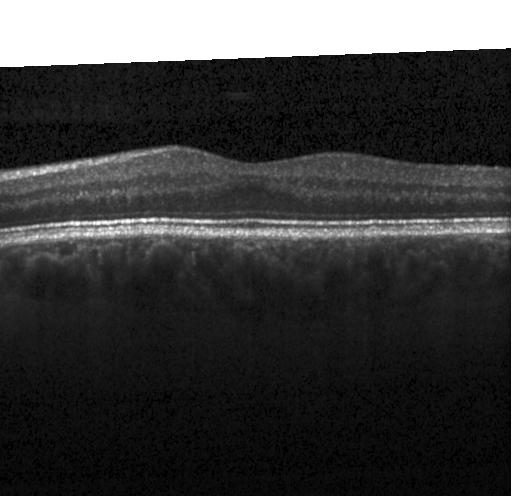
Macular scan, acquired on a Heidelberg Spectralis, optical coherence tomography B-scan — Finding: no CNV, no DME, and no drusen.